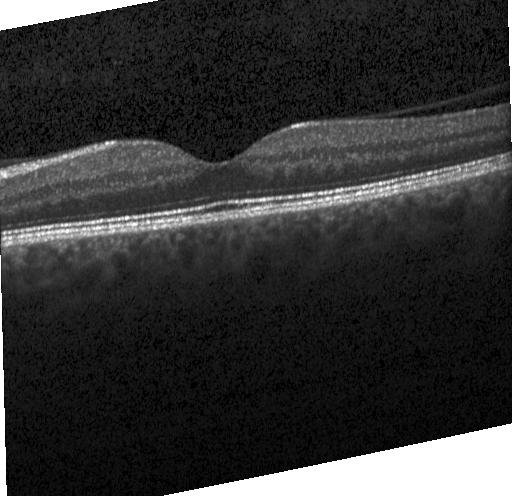
OCT B-scan. Impression: no choroidal neovascularization, diabetic macular edema, or drusen.